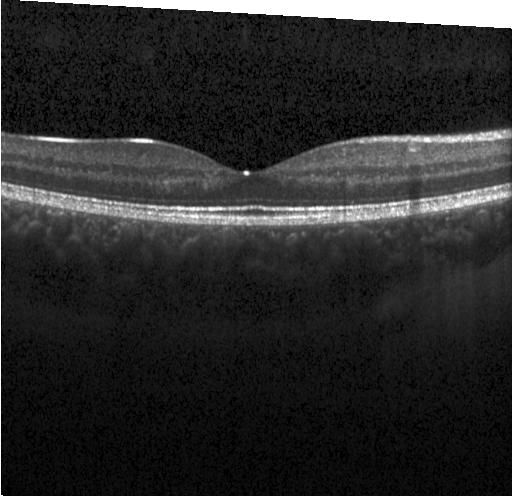

Instrument: Heidelberg Spectralis. OCT B-scan. SD-OCT. Macular scan.
The scan shows neither choroidal neovascularization, diabetic macular edema, nor drusen.